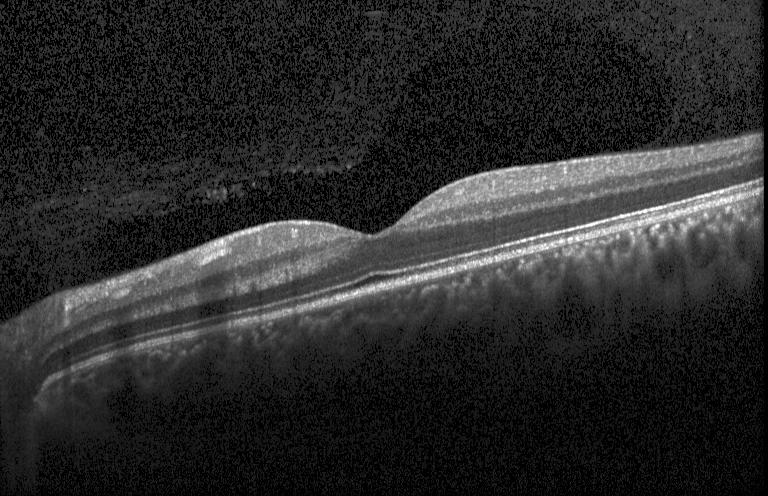 OCT finding: no choroidal neovascularization, no diabetic macular edema, and no drusen.